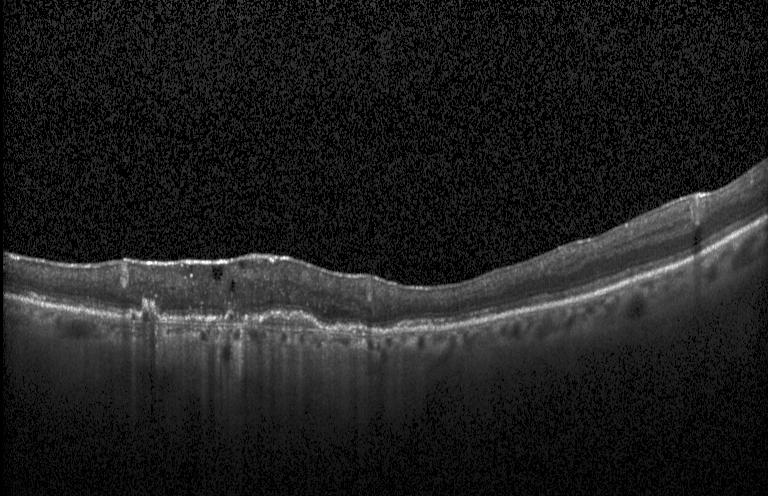 OCT line scan.
Impression: choroidal neovascularization (CNV).